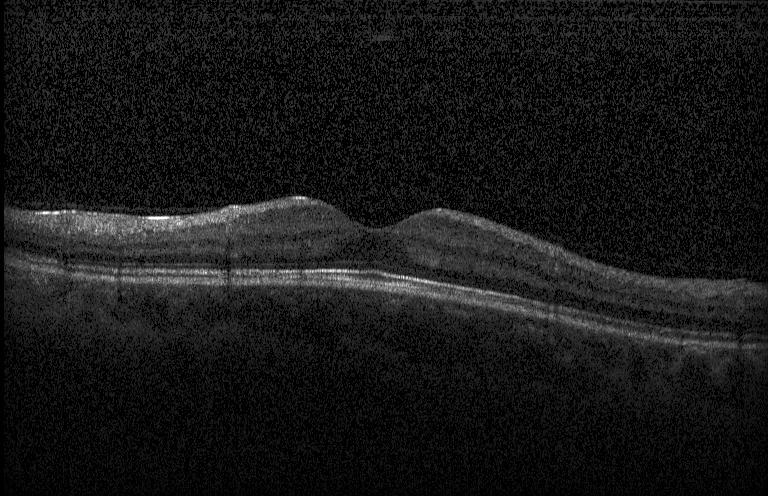
Retinal OCT B-scan. Assessment: no CNV, DME, or drusen.